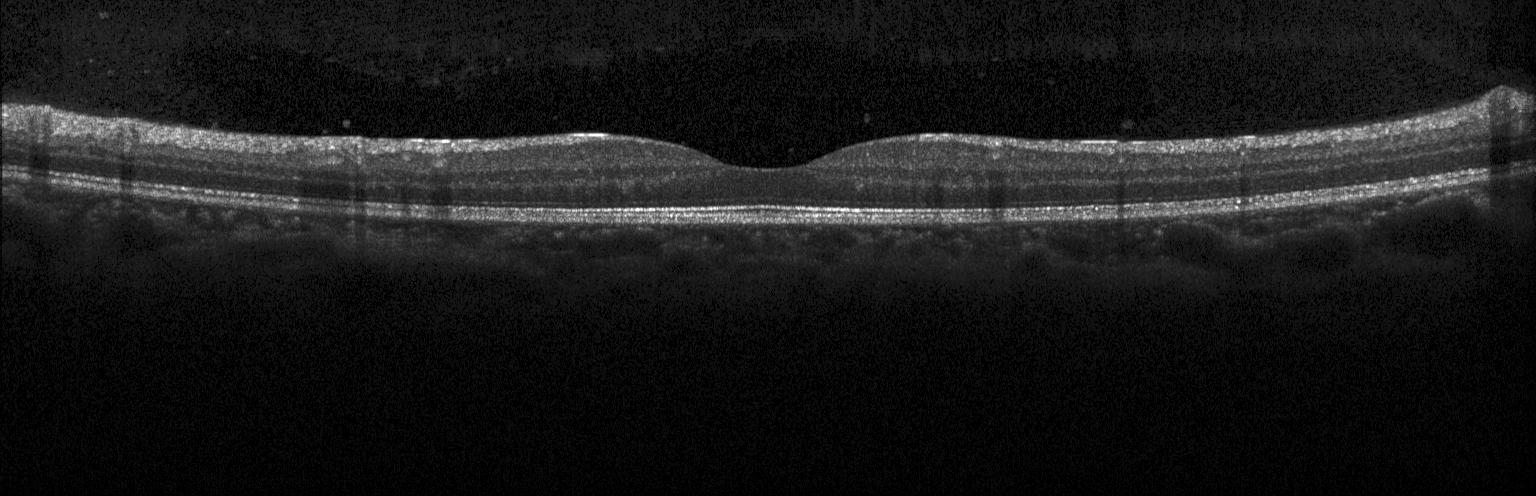

Assessment: no choroidal neovascularization, diabetic macular edema, or drusen.